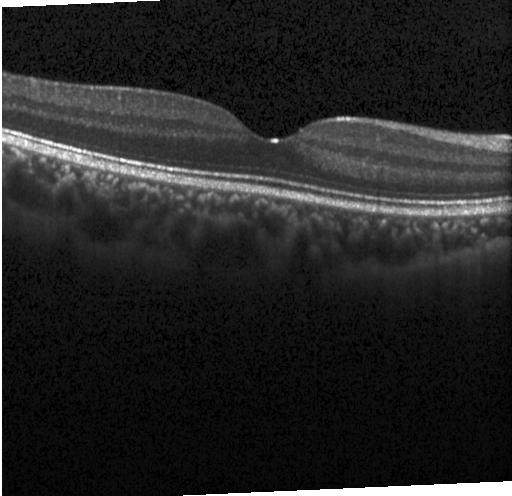
The scan shows no CNV, no DME, and no drusen.